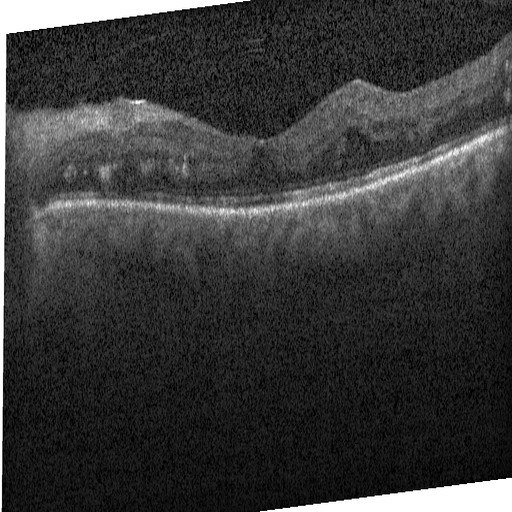 Optical coherence tomography B-scan.
Impression: diabetic macular edema.